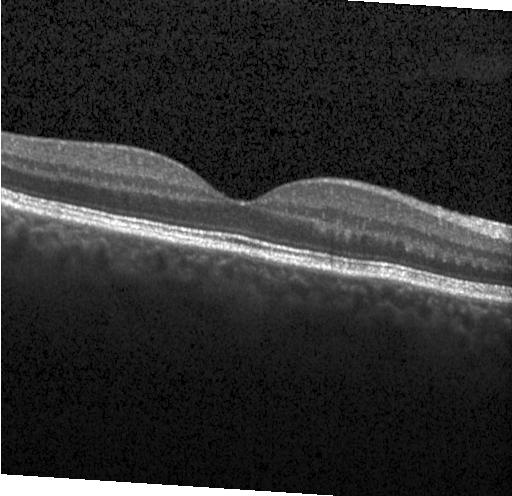
SD-OCT, macular scan, retinal OCT cross-section, instrument: Heidelberg Spectralis.
Dx: no choroidal neovascularization, no diabetic macular edema, and no drusen.